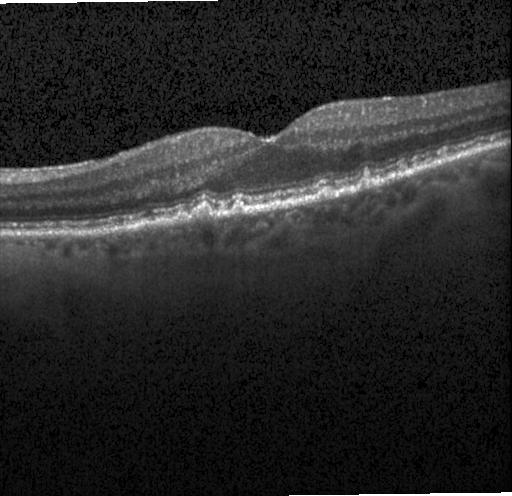
Dx: sub-RPE drusenoid deposits.